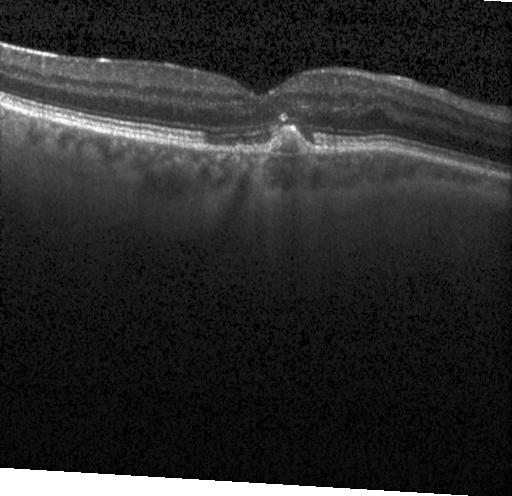

Horizontal scan through the fovea. Instrument: Heidelberg Spectralis. Spectral-domain optical coherence tomography. Optical coherence tomography scan.
Assessment: CNV.